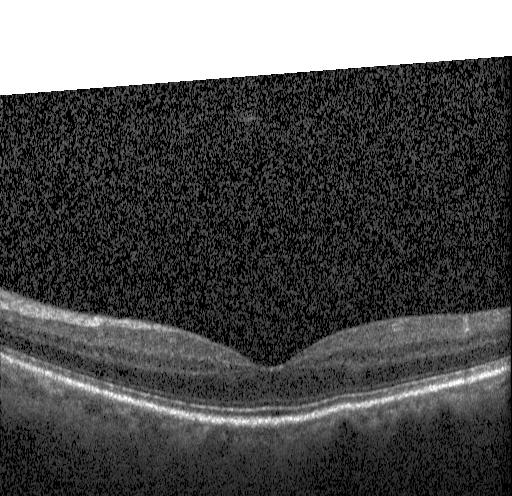 Dx: no CNV, DME, or drusen.